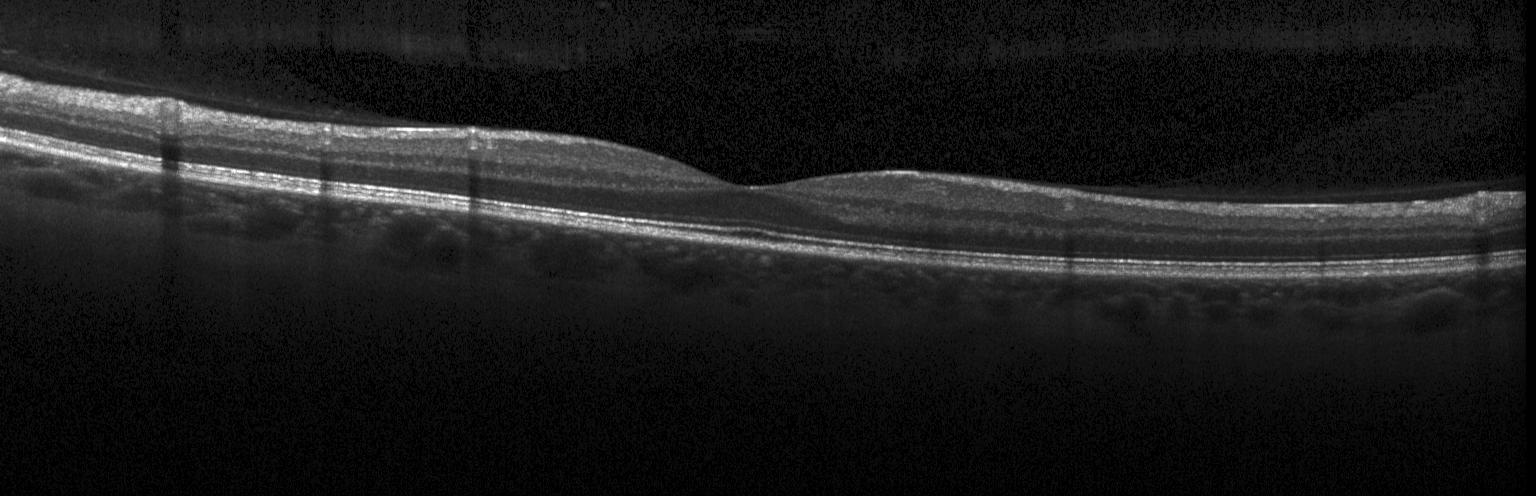

Fovea-centered, optical coherence tomography scan. Diagnosis: no CNV, no DME, and no drusen.